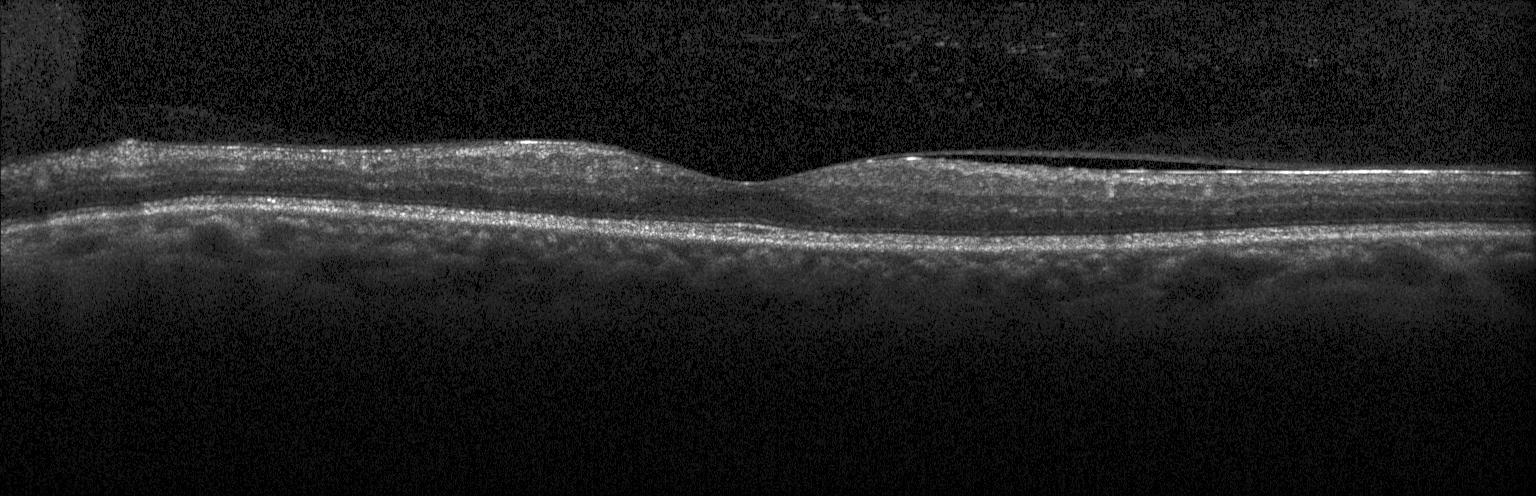
OCT scan showing diabetic macular edema.